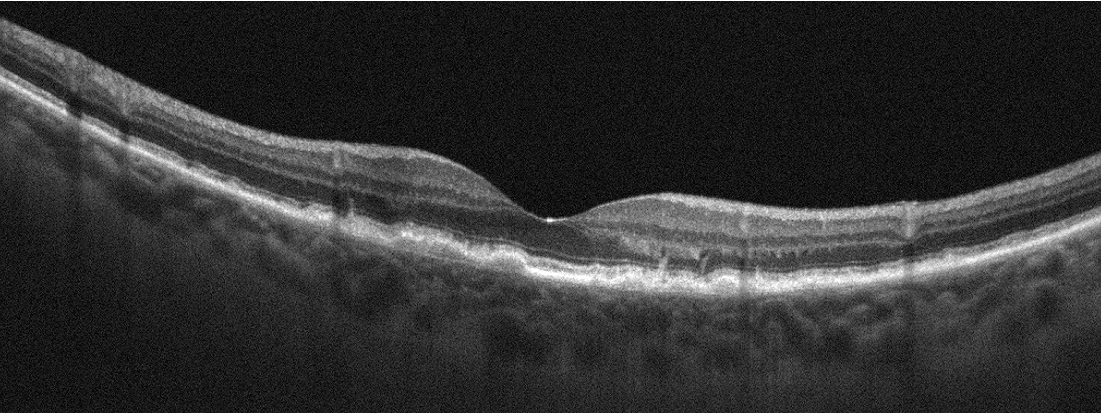 Fovea-centered; Optovue Avanti RTVue XR; retinal OCT cross-section. Finding: AMD.